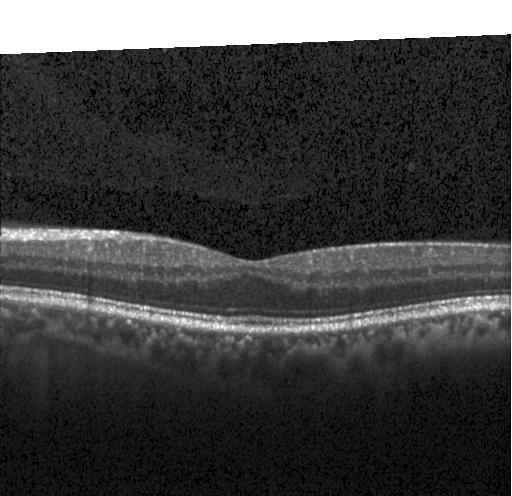
Horizontal scan through the fovea · acquired on a Heidelberg Spectralis · optical coherence tomography scan. OCT finding: no evidence of choroidal neovascularization, diabetic macular edema, or drusen.